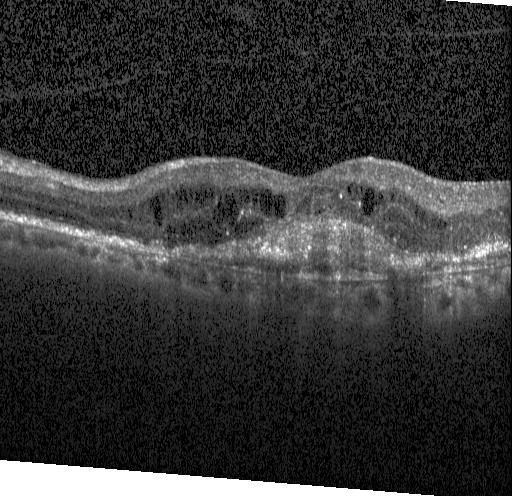

OCT B-scan showing CNV.